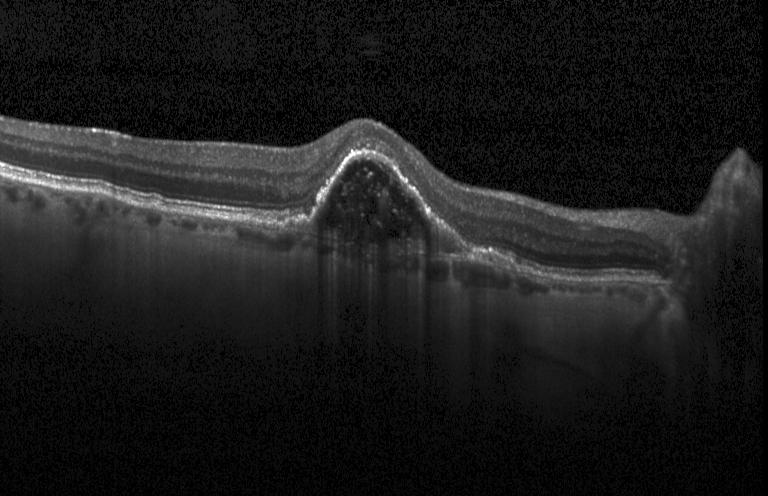
Retinal OCT cross-section
Diagnosis: choroidal neovascularization.